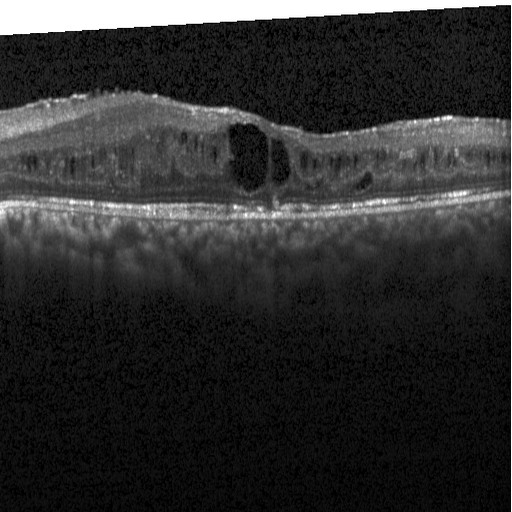 OCT B-scan
Diagnosis: diabetic macular edema (DME).